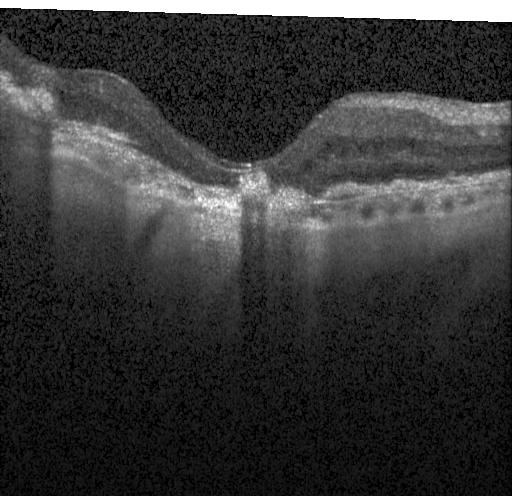
OCT B-scan. Heidelberg Spectralis. Centered on the fovea. Spectral-domain optical coherence tomography — Impression: a choroidal neovascular membrane.